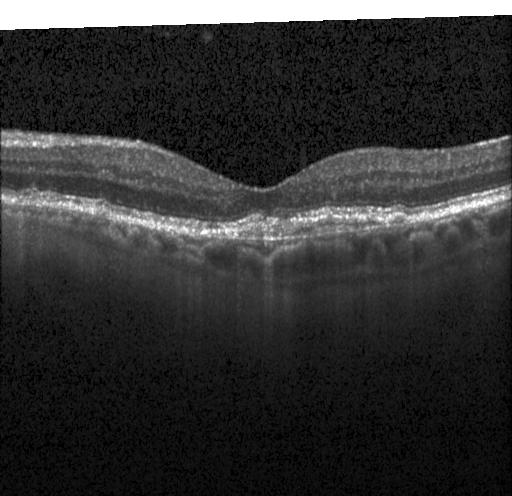

Dx: a choroidal neovascular membrane.